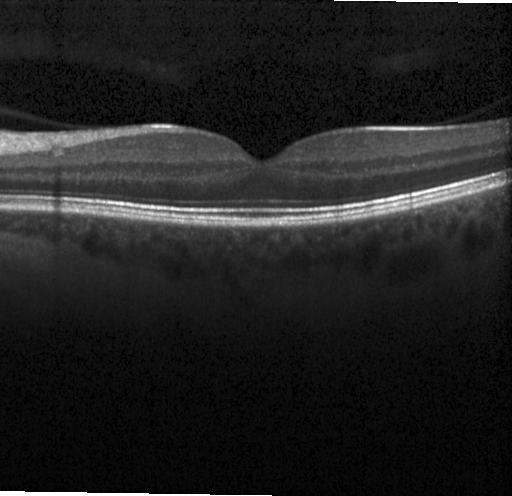

Retinal OCT B-scan.
OCT finding: neither CNV, DME, nor drusen.